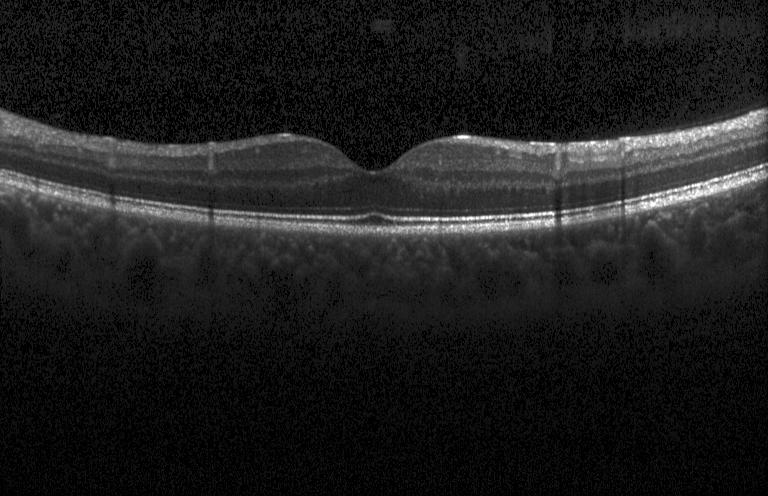

Optical coherence tomography B-scan.
Dx: no evidence of choroidal neovascularization, diabetic macular edema, or drusen.